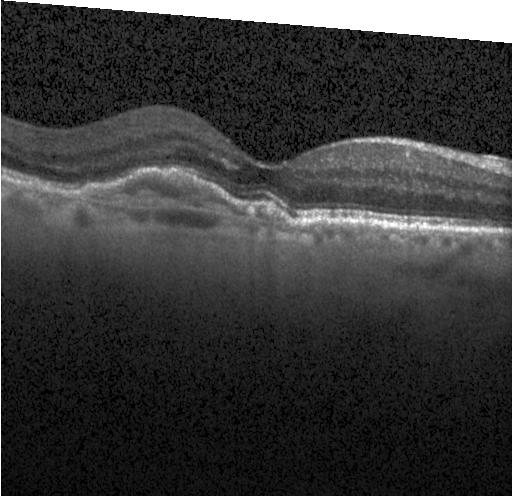
Heidelberg Spectralis OCT system, retinal OCT cross-section
A choroidal neovascular membrane.